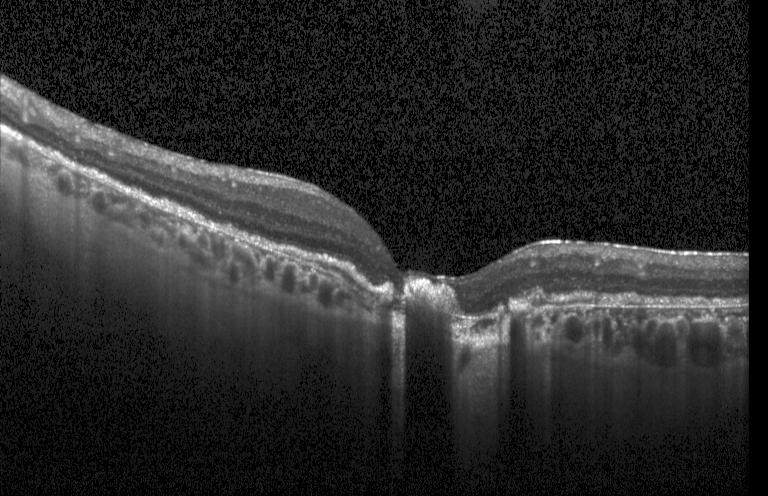
OCT B-scan · through the macula · Heidelberg Spectralis OCT system.
Impression: a choroidal neovascular membrane.